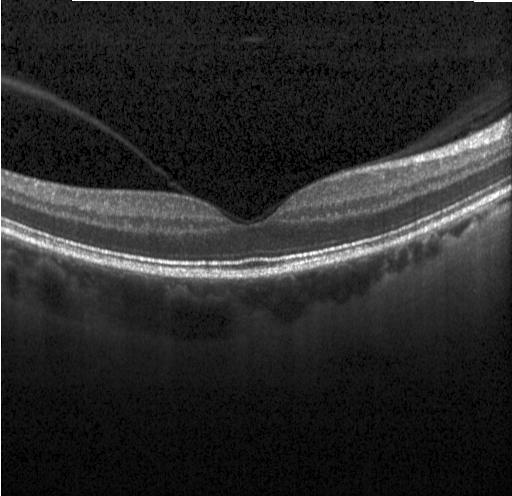 Retinal OCT cross-section
Dx: no choroidal neovascularization, diabetic macular edema, or drusen.